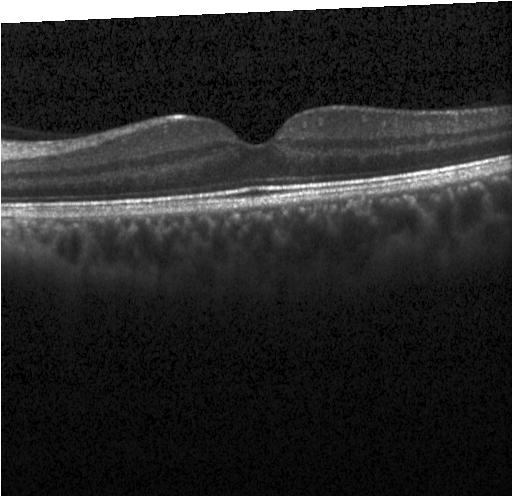 SD-OCT. Retinal OCT B-scan — Finding: no evidence of choroidal neovascularization, diabetic macular edema, or drusen.